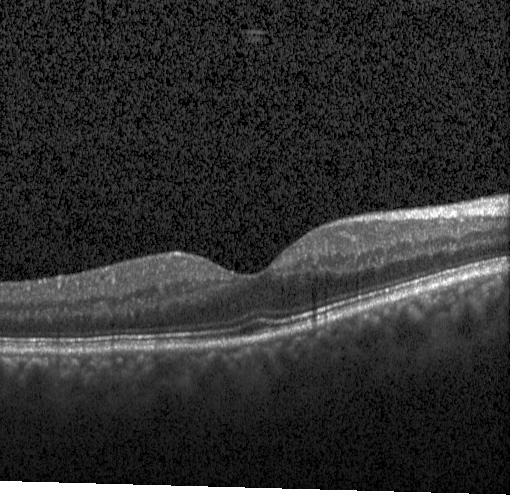
Optical coherence tomography B-scan.
Neither choroidal neovascularization, diabetic macular edema, nor drusen.